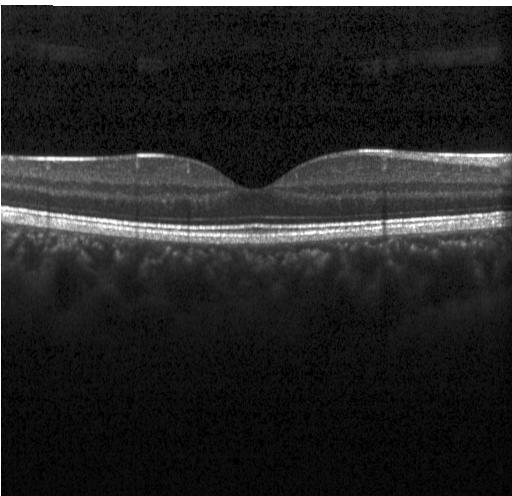 OCT finding: neither choroidal neovascularization, diabetic macular edema, nor drusen.